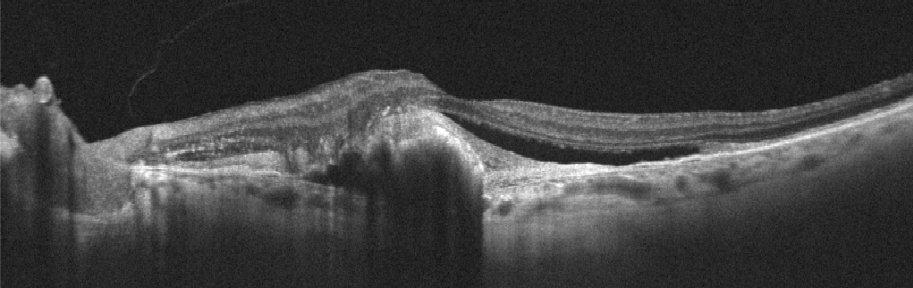
Optical coherence tomography B-scan · acquired on an Optovue Avanti RTVue XR
Age-related macular degeneration.